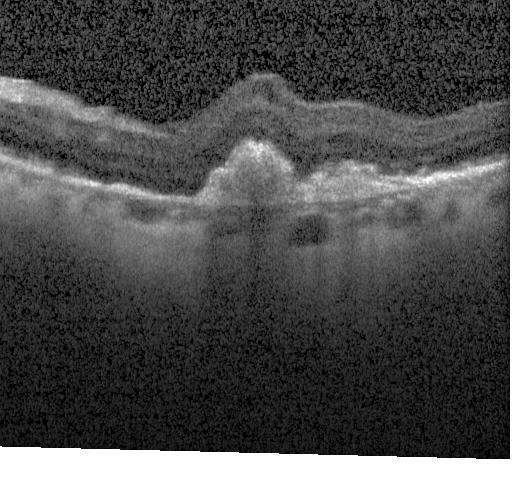 Retinal OCT cross-section showing CNV.